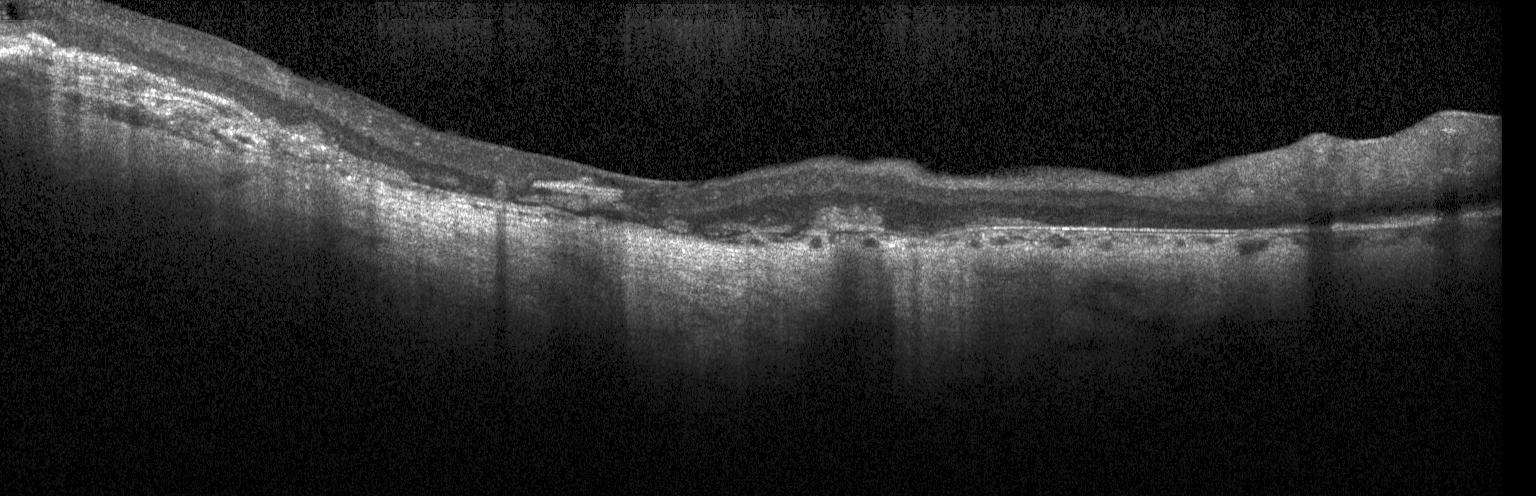

Impression: choroidal neovascularization.